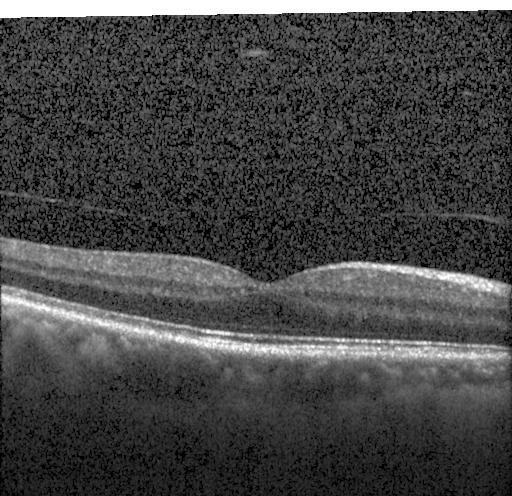
Retinal OCT B-scan; acquired on a Heidelberg Spectralis; spectral-domain OCT — Assessment: no CNV, DME, or drusen.